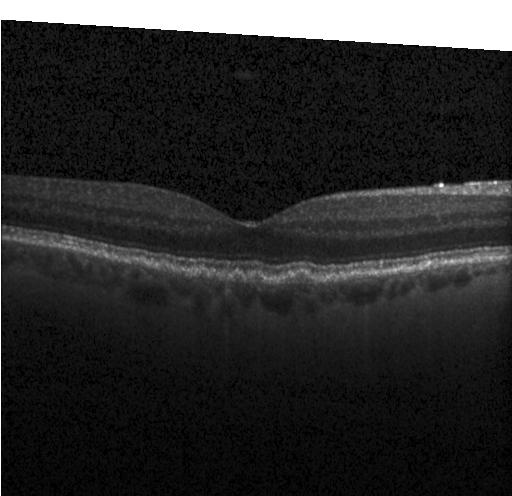
OCT finding: sub-RPE drusenoid deposits.